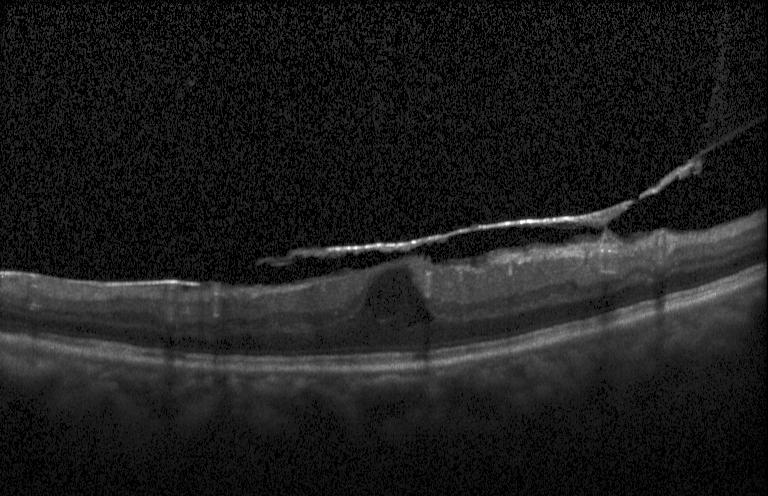
Finding: diabetic macular edema (DME).